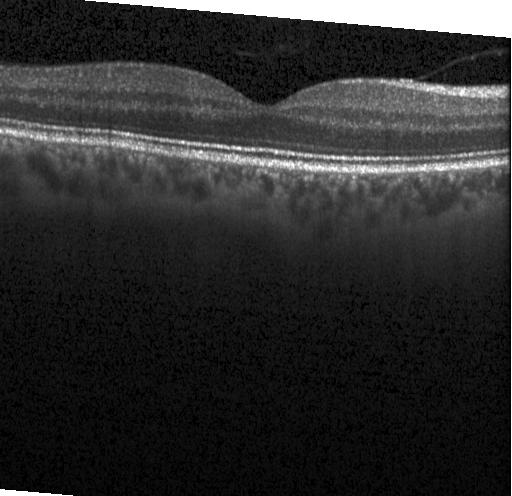
OCT B-scan. Finding: neither CNV, DME, nor drusen.